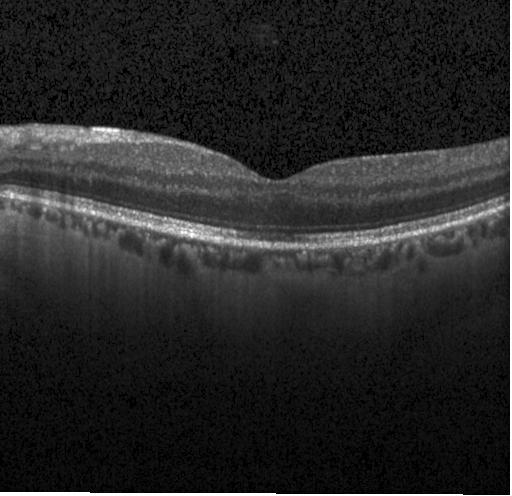 Retinal OCT cross-section
Diagnosis: neither CNV, DME, nor drusen.